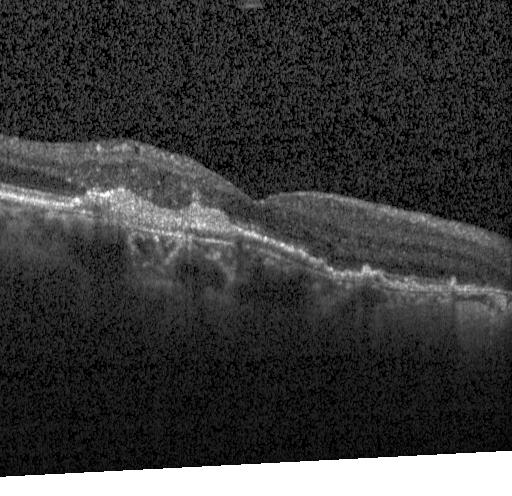 This B-scan demonstrates a choroidal neovascular membrane.